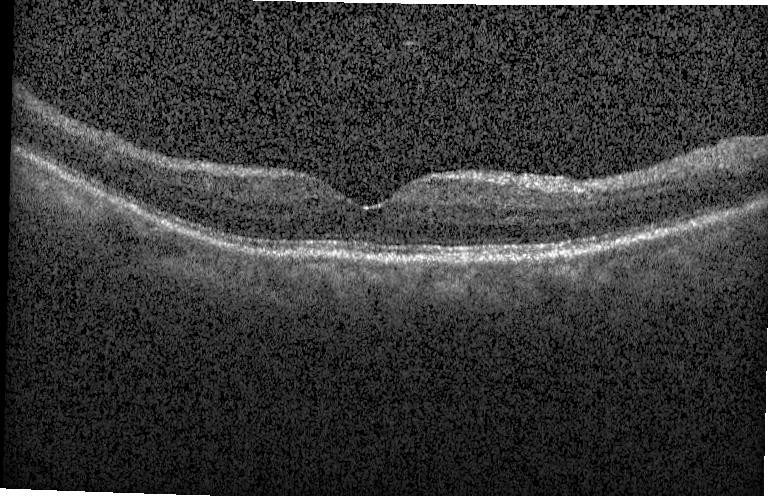
Retinal OCT cross-section.
Finding: no CNV, no DME, and no drusen.